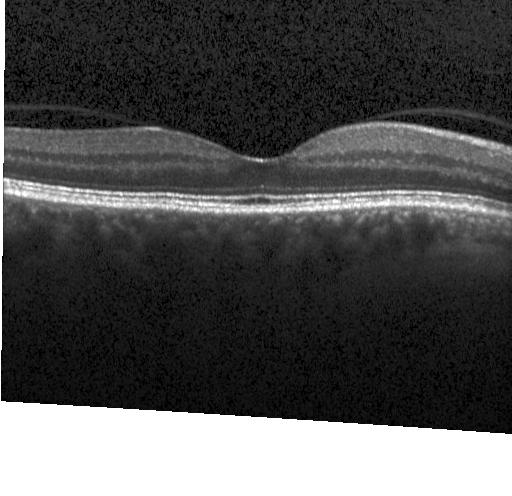 Acquired on a Heidelberg Spectralis, OCT B-scan, centered on the fovea, spectral-domain OCT
This B-scan demonstrates no evidence of choroidal neovascularization, diabetic macular edema, or drusen.